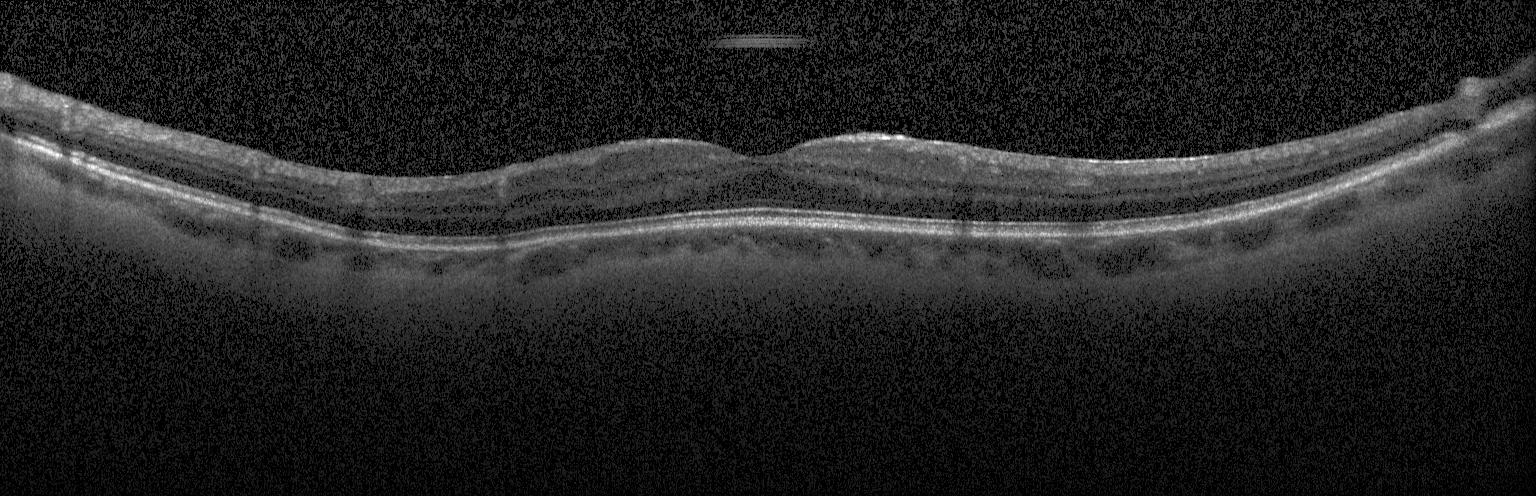 Diagnosis: neither CNV, DME, nor drusen.